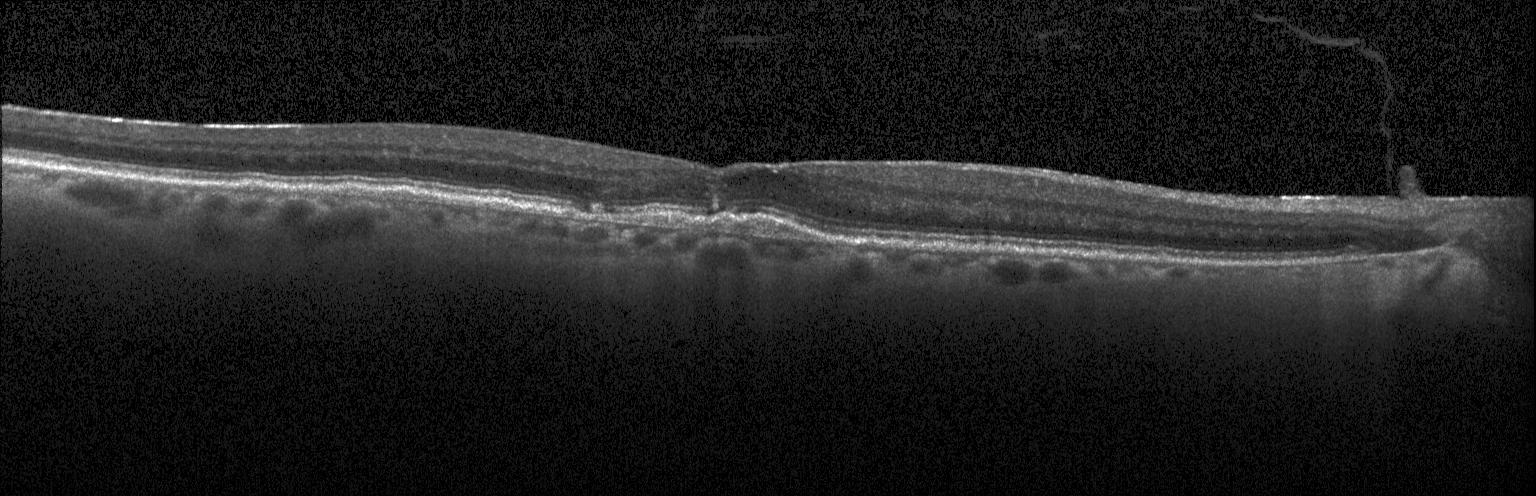

OCT B-scan. Impression: a choroidal neovascular membrane.